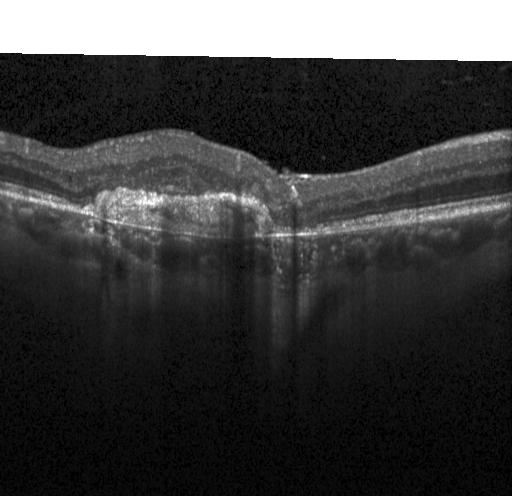

Spectral-domain OCT B-scan: a choroidal neovascular membrane.